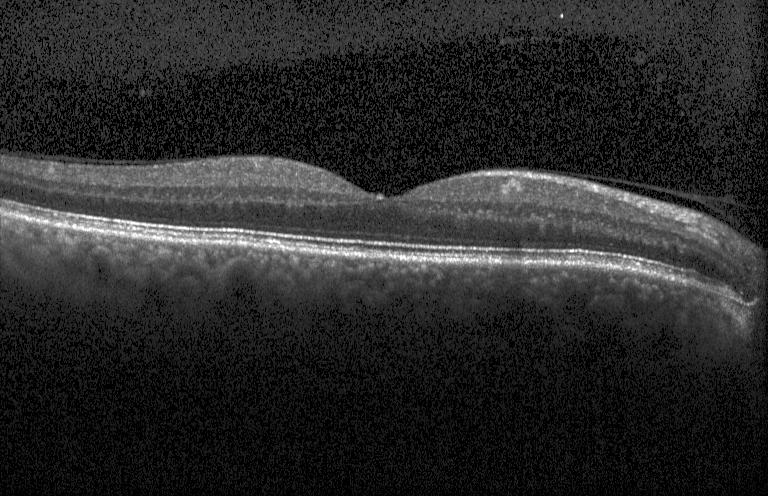
Impression: no evidence of choroidal neovascularization, diabetic macular edema, or drusen.